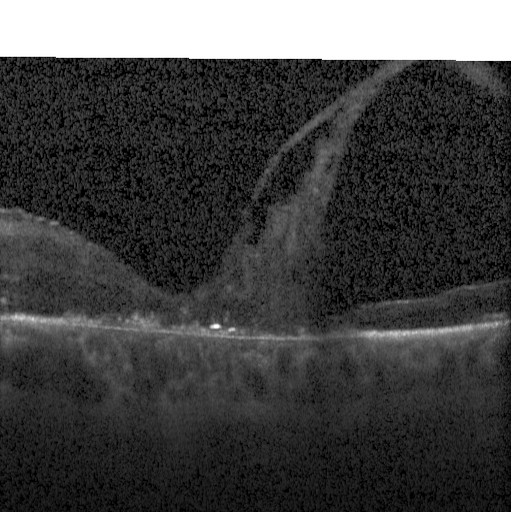

Centered on the fovea; Heidelberg Spectralis OCT system; optical coherence tomography scan; spectral-domain optical coherence tomography — Diagnosis: DME.